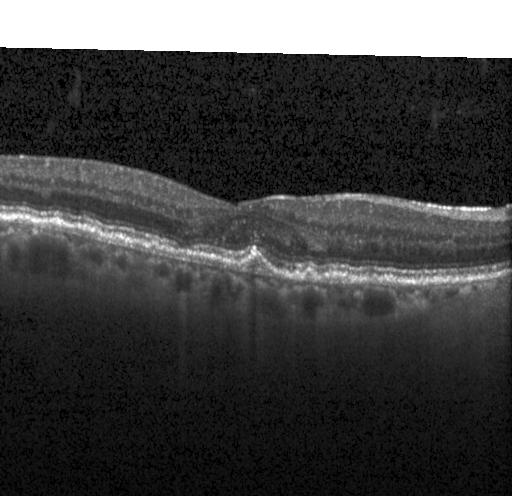
OCT B-scan.
Diagnosis: drusen.